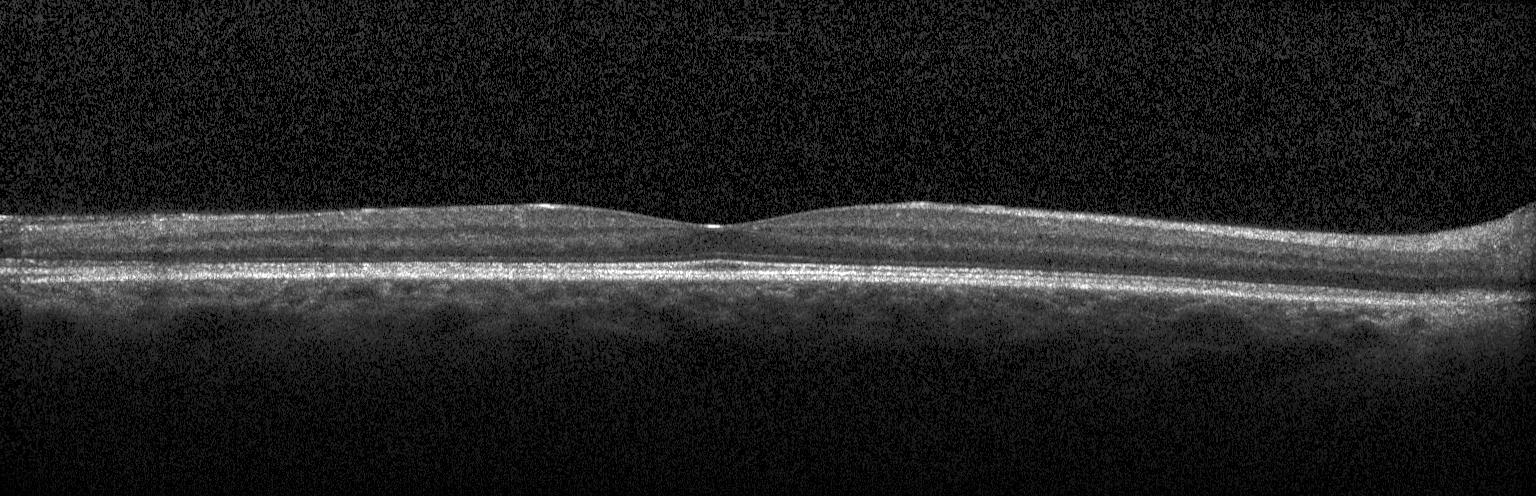
Optical coherence tomography scan · instrument: Heidelberg Spectralis
Impression: no evidence of choroidal neovascularization, diabetic macular edema, or drusen.